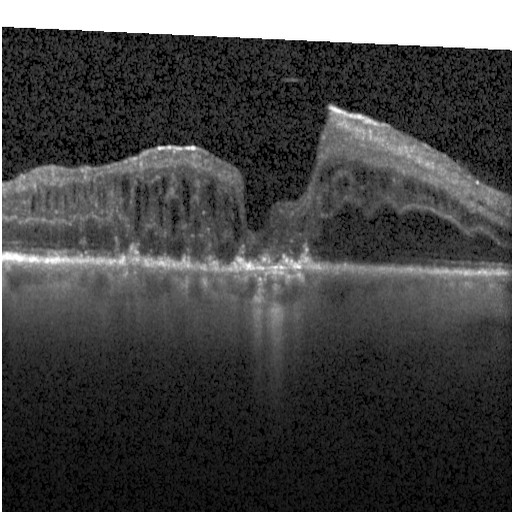 OCT line scan, horizontal scan through the fovea. Macular OCT: diabetic macular edema.